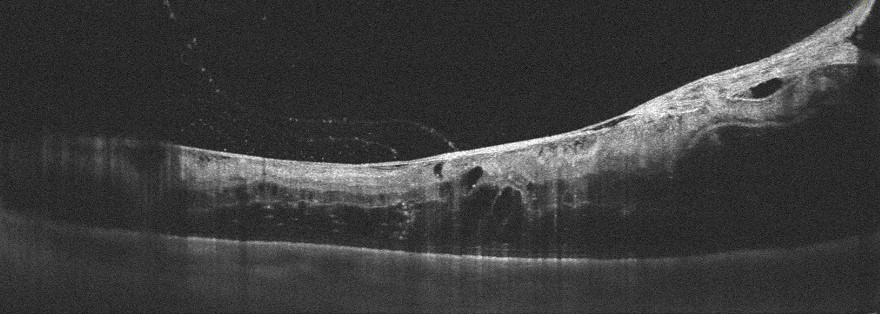

Macular scan · instrument: Optovue Avanti RTVue XR · retinal OCT B-scan.
Impression: diabetic macular edema.